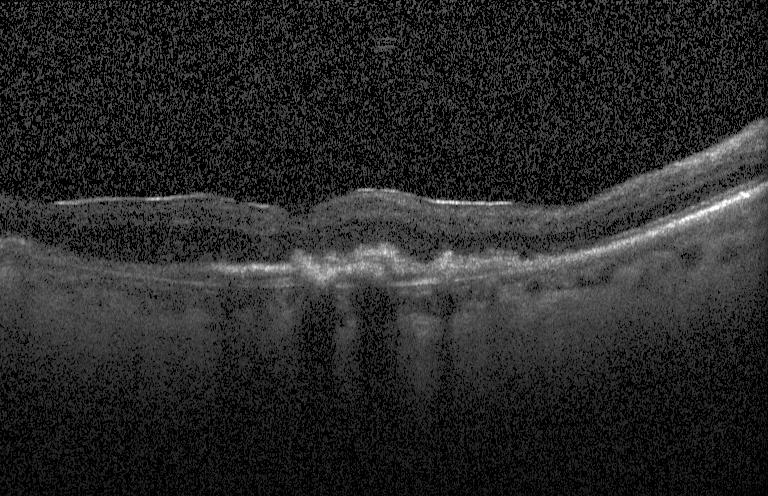

OCT line scan.
Dx: choroidal neovascularization (CNV).